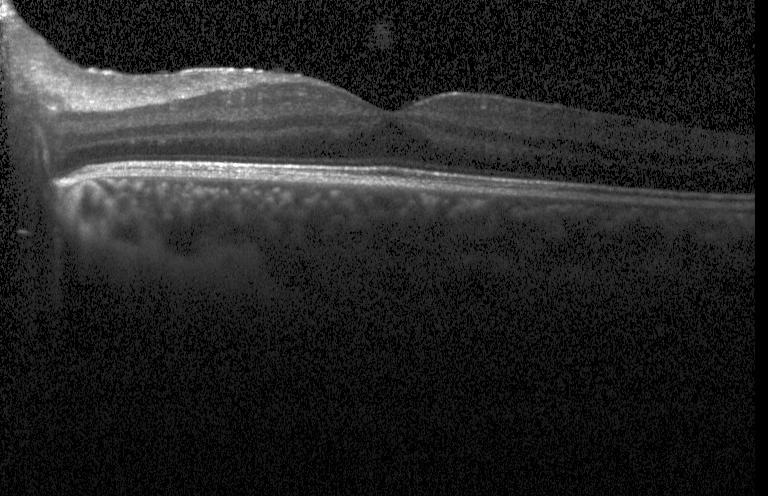 Acquired on a Heidelberg Spectralis. Optical coherence tomography B-scan. Centered on the fovea.
Assessment: neither choroidal neovascularization, diabetic macular edema, nor drusen.